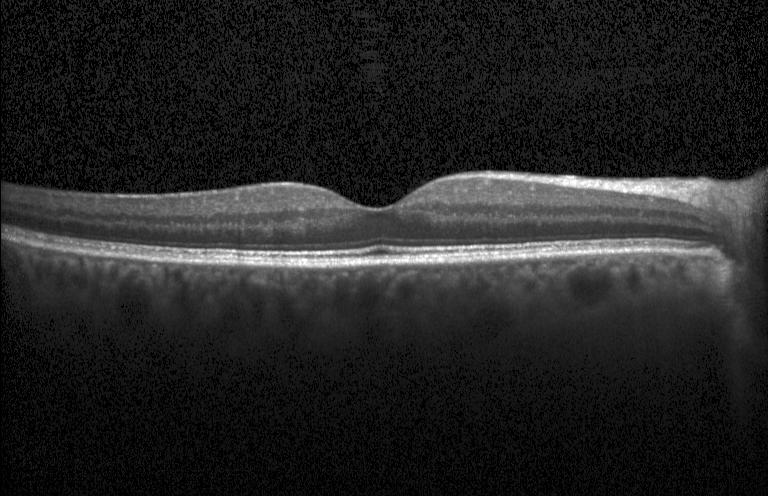

Optical coherence tomography scan · spectral-domain OCT. Diagnosis: no choroidal neovascularization, diabetic macular edema, or drusen.